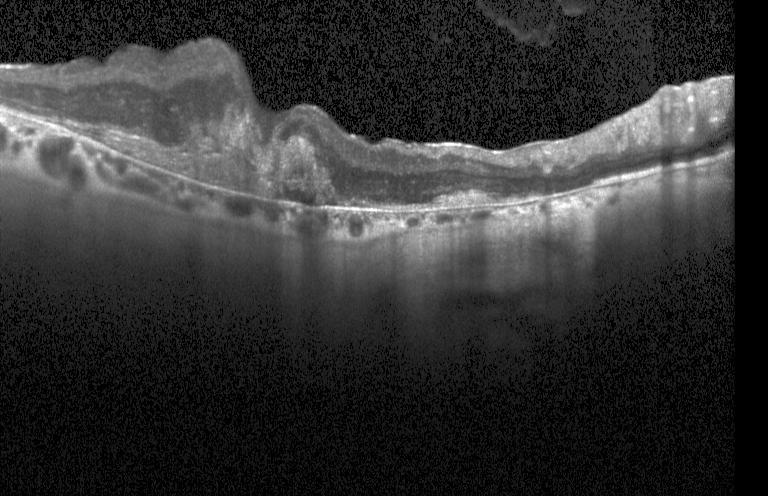

Optical coherence tomography B-scan — OCT finding: choroidal neovascularization.